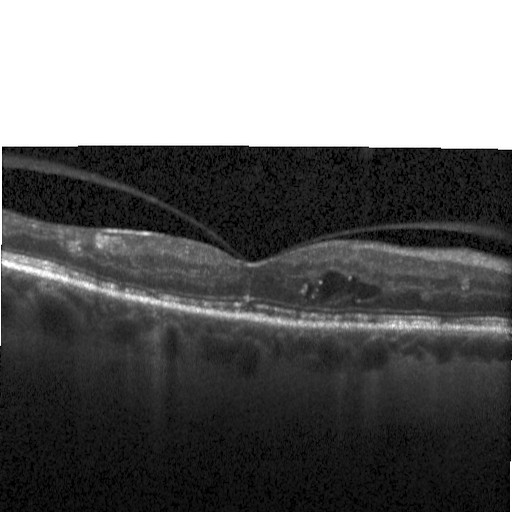

Through the macula. Retinal OCT B-scan. SD-OCT. Heidelberg Spectralis OCT system — Impression: diabetic macular edema (DME).